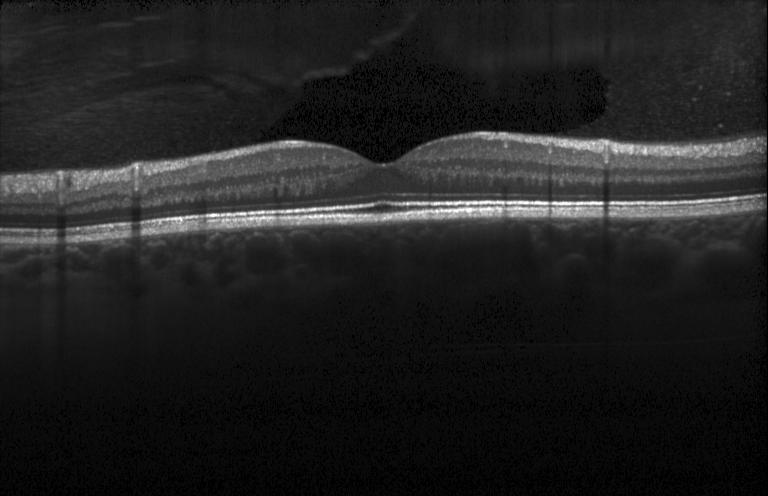

The scan shows no choroidal neovascularization, no diabetic macular edema, and no drusen.